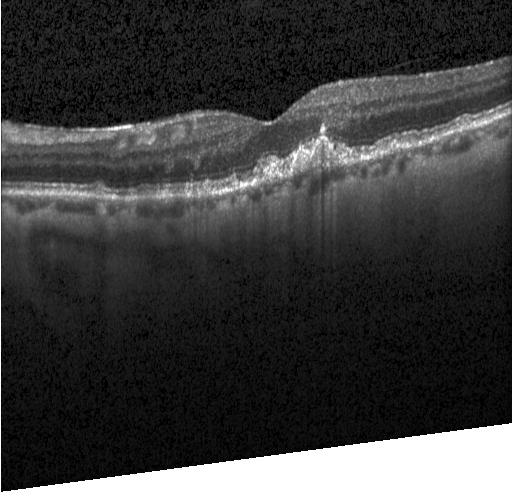
Assessment: a choroidal neovascular membrane.